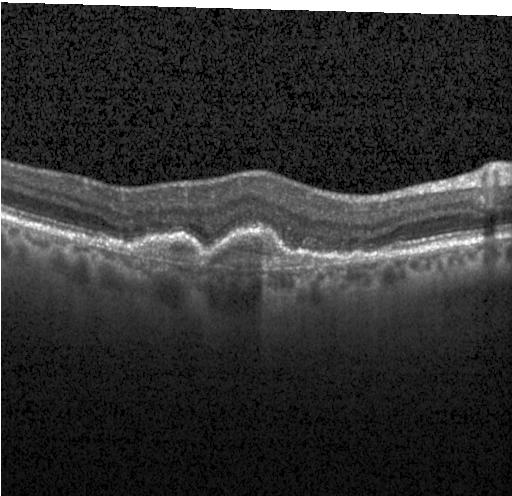 Spectral-domain optical coherence tomography, optical coherence tomography scan, Heidelberg Spectralis OCT system — Impression: choroidal neovascularization.